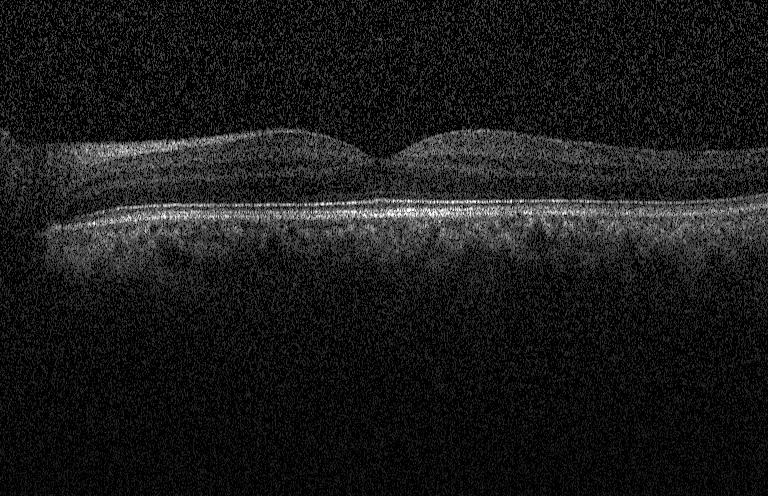
Retinal OCT B-scan, fovea-centered, acquired on a Heidelberg Spectralis, spectral-domain optical coherence tomography — Macular OCT: neither choroidal neovascularization, diabetic macular edema, nor drusen.